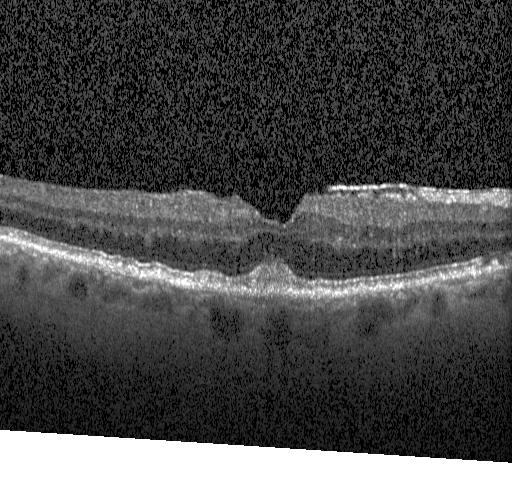 OCT finding: sub-RPE drusenoid deposits.